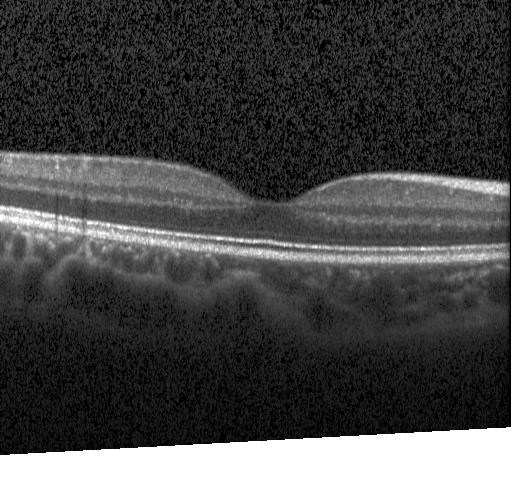
Impression: no choroidal neovascularization, no diabetic macular edema, and no drusen.